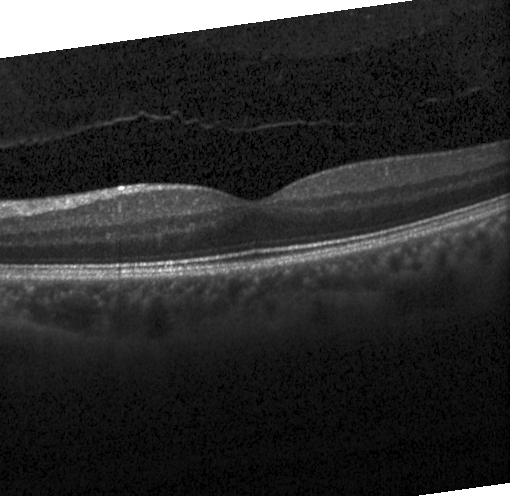
Retinal OCT cross-section showing no choroidal neovascularization, no diabetic macular edema, and no drusen.